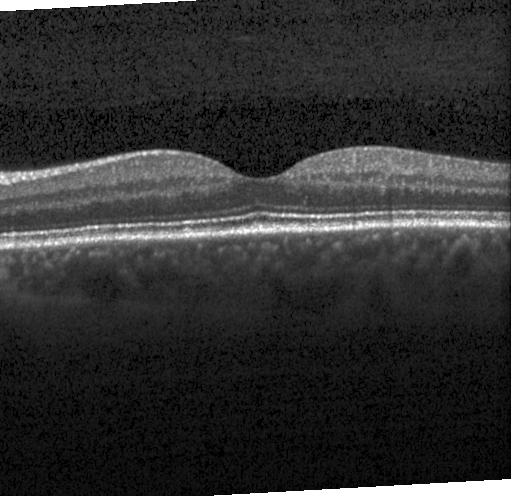

Instrument: Heidelberg Spectralis, macular scan, OCT B-scan.
Finding: neither CNV, DME, nor drusen.